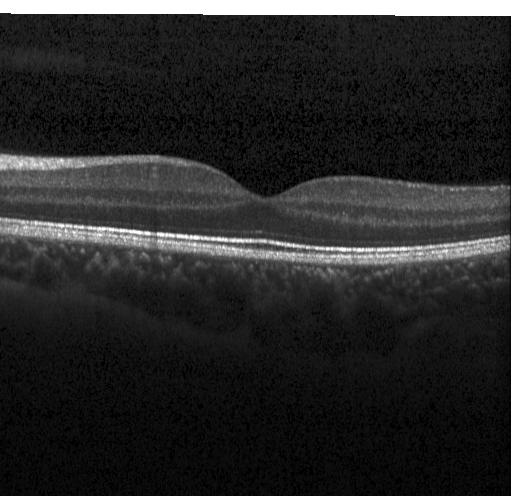
Macular OCT: neither CNV, DME, nor drusen.